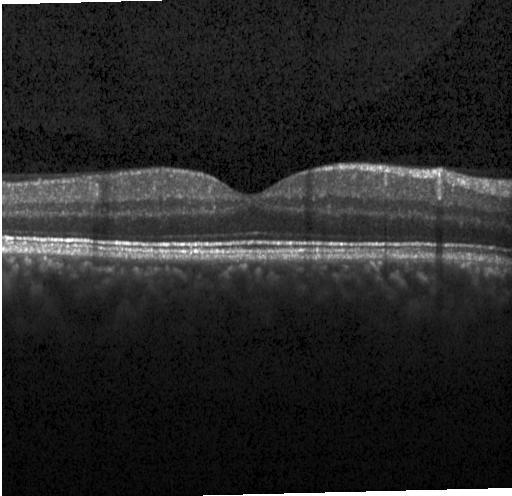 Optical coherence tomography scan, Heidelberg Spectralis. Macular OCT: no CNV, DME, or drusen.